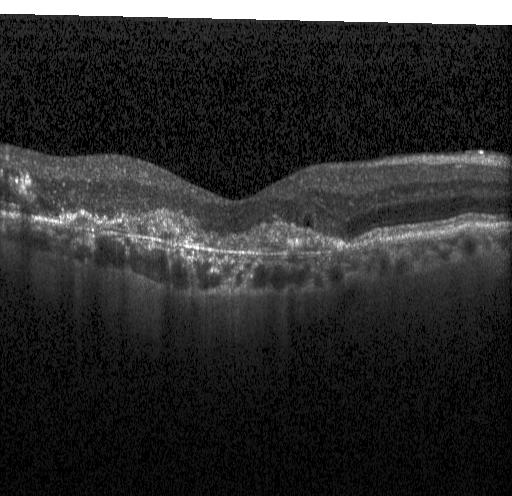

Optical coherence tomography scan; acquired on a Heidelberg Spectralis — Diagnosis: a choroidal neovascular membrane.